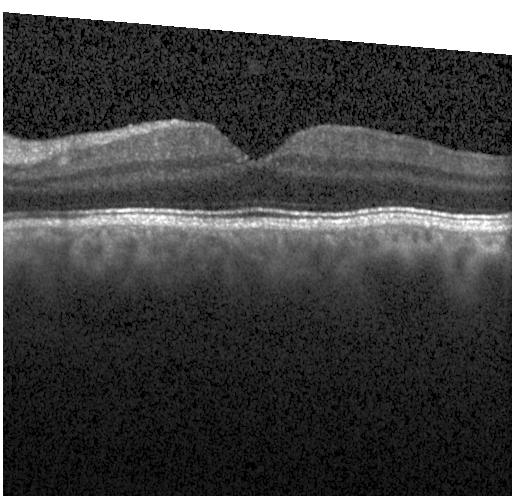

Spectral-domain OCT B-scan: no evidence of choroidal neovascularization, diabetic macular edema, or drusen.